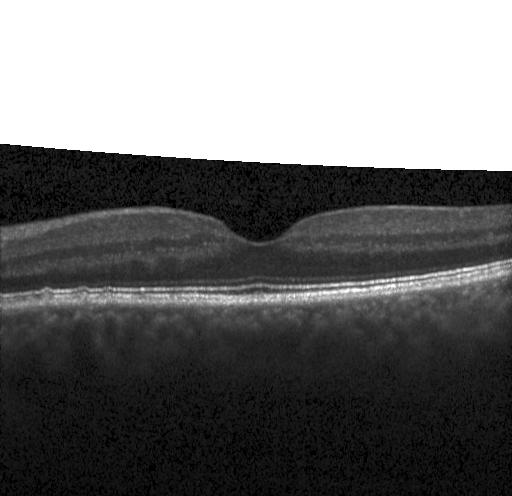
Heidelberg Spectralis; retinal OCT cross-section; SD-OCT; through the macula
Macular OCT: no evidence of choroidal neovascularization, diabetic macular edema, or drusen.